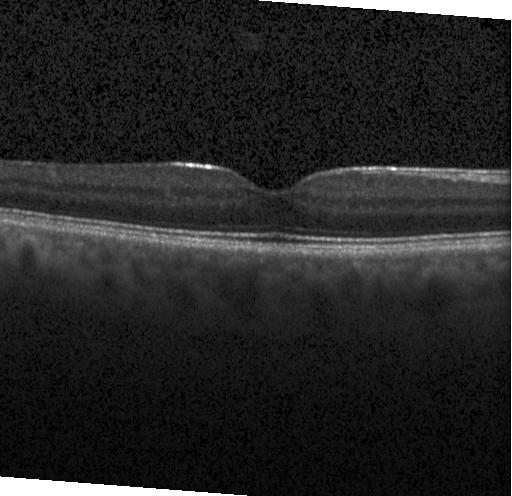 OCT line scan; spectral-domain OCT
Impression: no evidence of choroidal neovascularization, diabetic macular edema, or drusen.